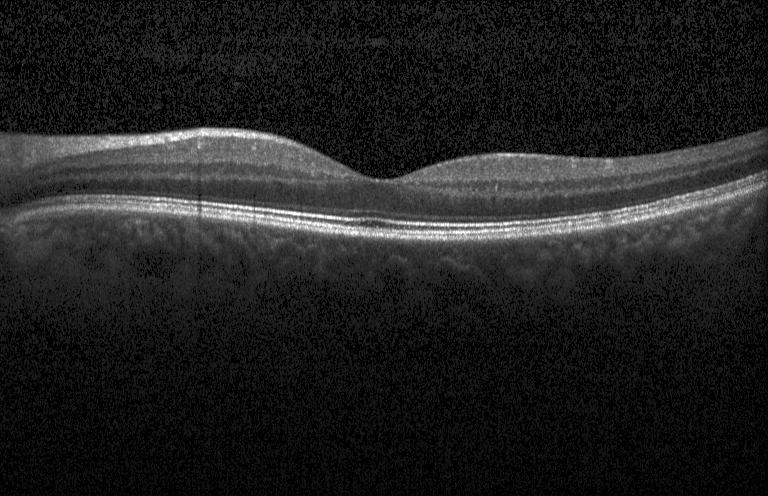 Finding: neither choroidal neovascularization, diabetic macular edema, nor drusen.